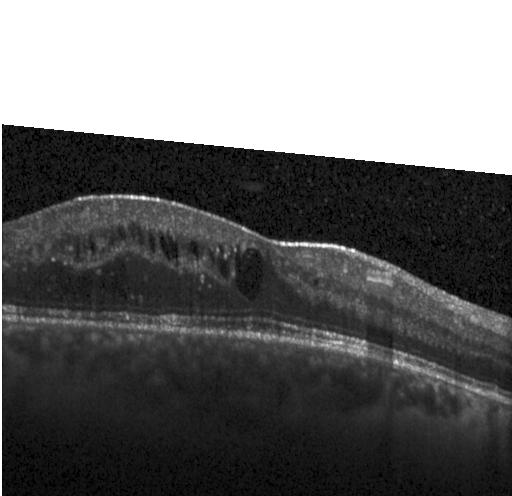
Spectral-domain OCT; horizontal scan through the fovea; Heidelberg Spectralis OCT system; optical coherence tomography B-scan
Impression: diabetic macular edema (DME).